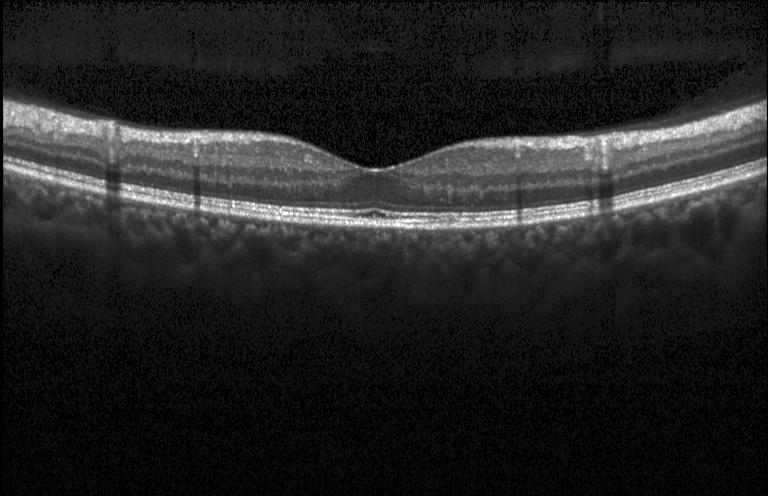
Spectral-domain OCT B-scan: no evidence of choroidal neovascularization, diabetic macular edema, or drusen.